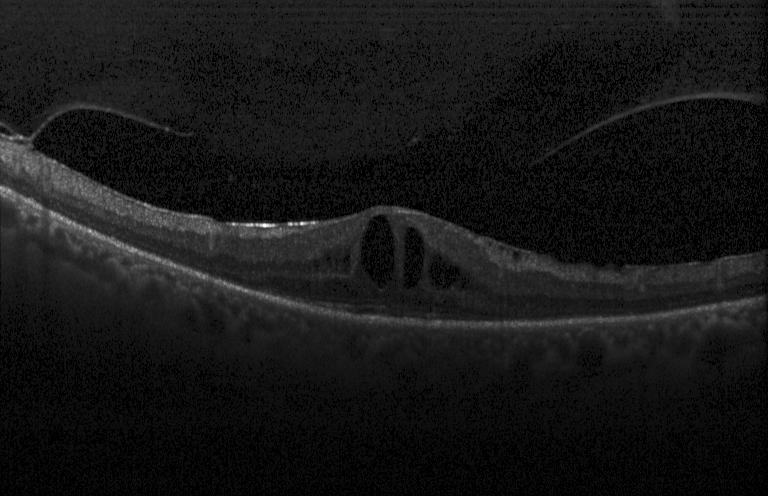
SD-OCT; Heidelberg Spectralis OCT system; OCT line scan
Diagnosis: DME.